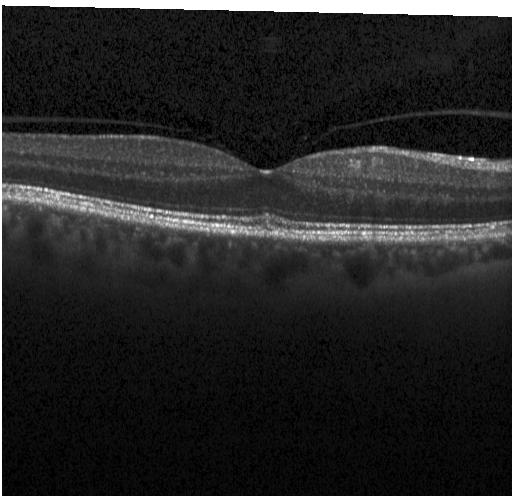
OCT B-scan; through the macula. This B-scan demonstrates no CNV, no DME, and no drusen.